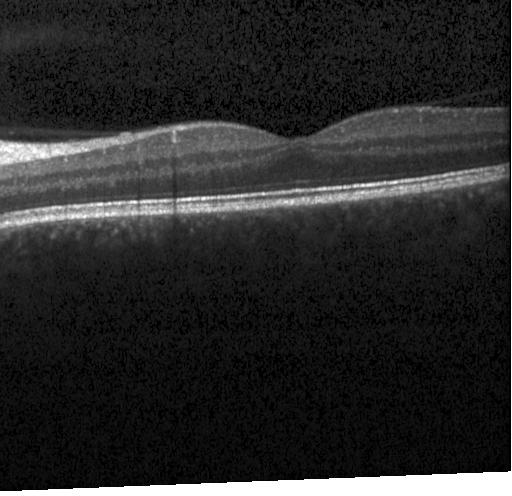
Optical coherence tomography B-scan; fovea-centered; spectral-domain OCT.
Impression: no choroidal neovascularization, no diabetic macular edema, and no drusen.